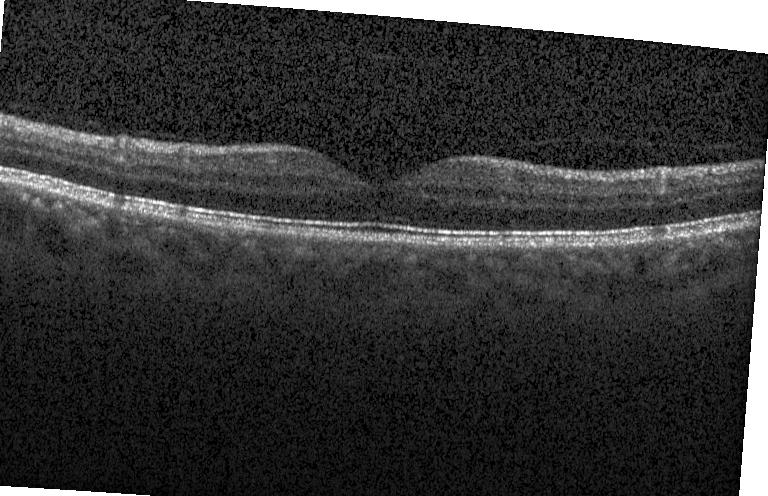

No evidence of choroidal neovascularization, diabetic macular edema, or drusen.